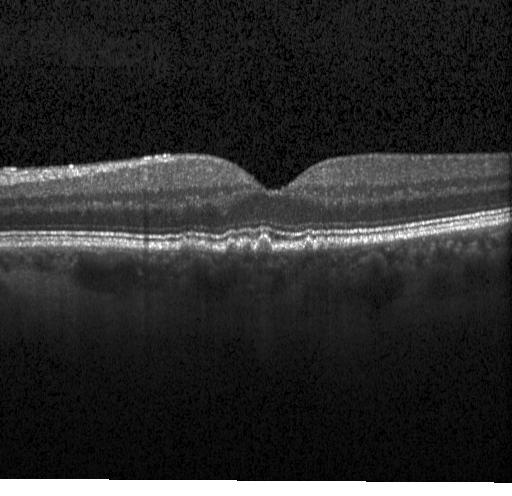

OCT B-scan showing sub-RPE drusenoid deposits.